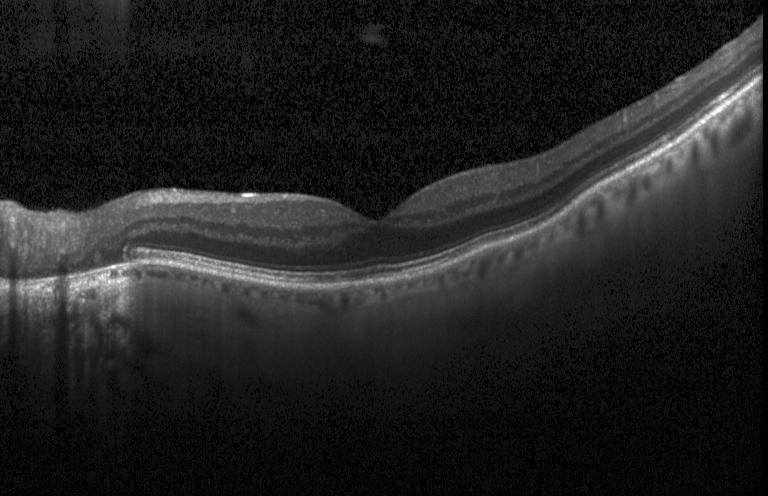
OCT line scan — Dx: no evidence of choroidal neovascularization, diabetic macular edema, or drusen.